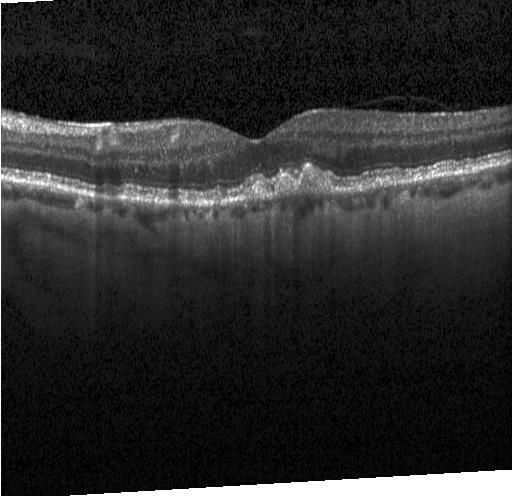
Instrument: Heidelberg Spectralis; OCT B-scan. This B-scan demonstrates drusen.